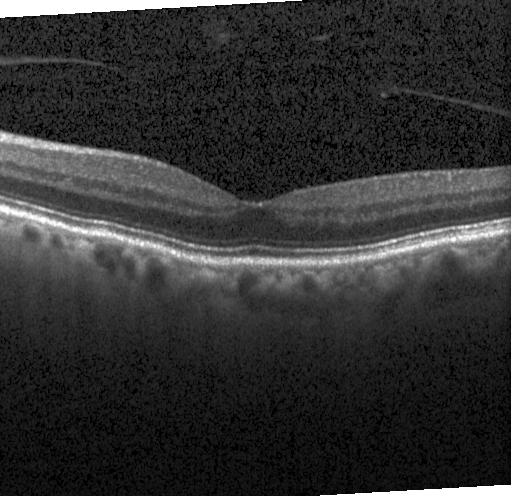 This B-scan demonstrates neither choroidal neovascularization, diabetic macular edema, nor drusen.